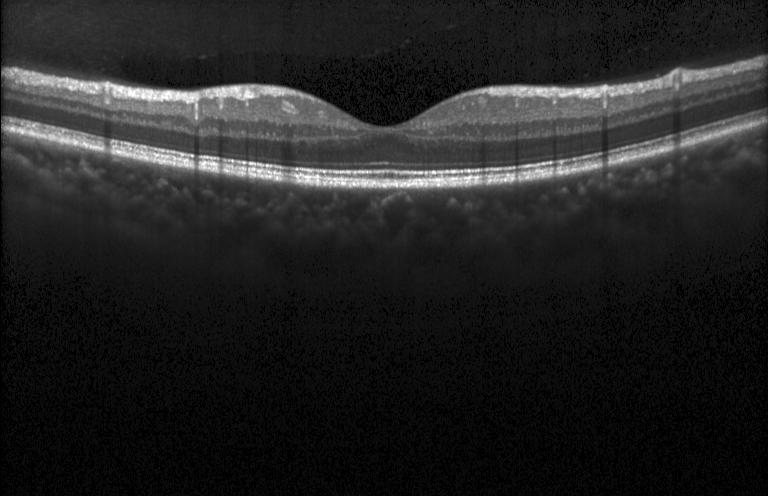

Retinal OCT B-scan. Fovea-centered
Diagnosis: no evidence of choroidal neovascularization, diabetic macular edema, or drusen.